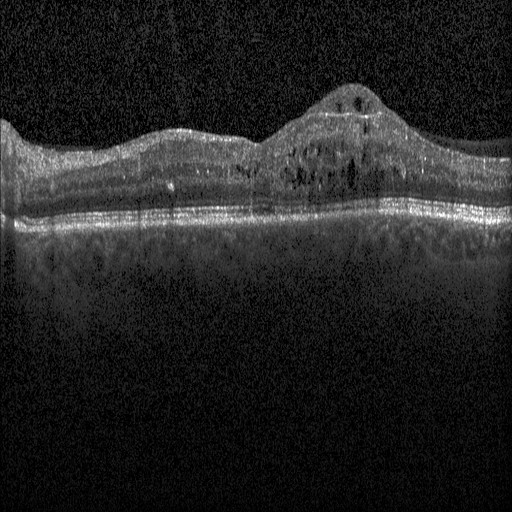 Diabetic macular edema.